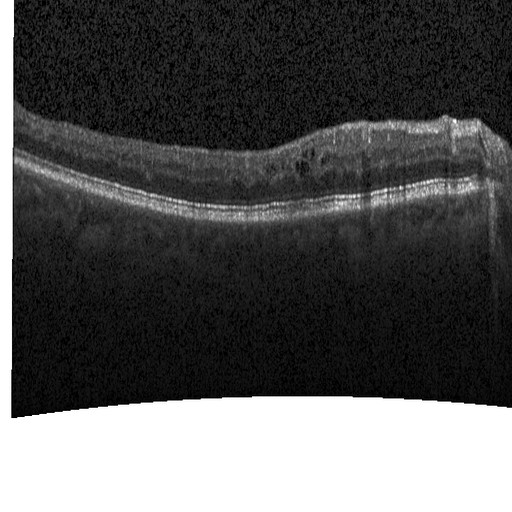

Retinal OCT cross-section
The scan shows DME.